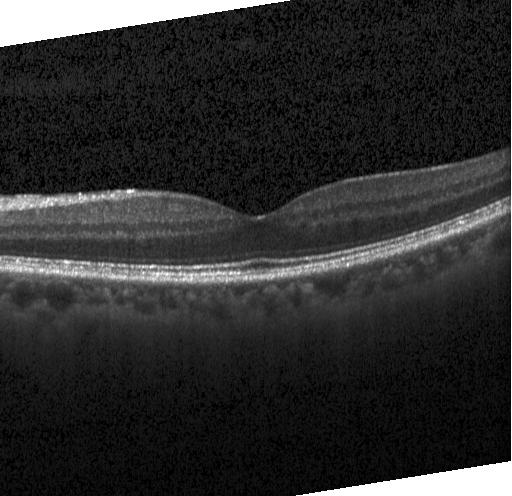

Heidelberg Spectralis, optical coherence tomography scan, spectral-domain OCT — Assessment: no choroidal neovascularization, diabetic macular edema, or drusen.